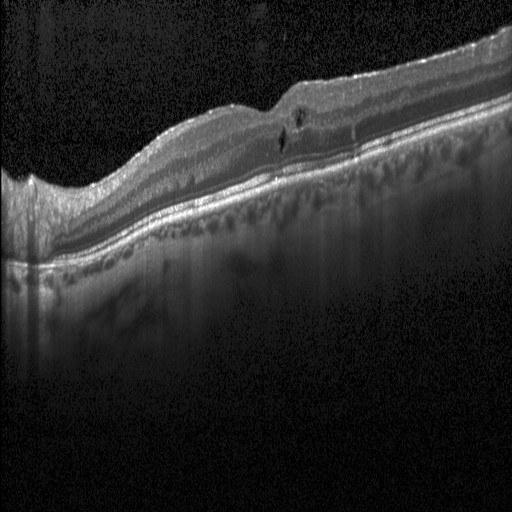
Macular OCT: diabetic macular edema (DME).